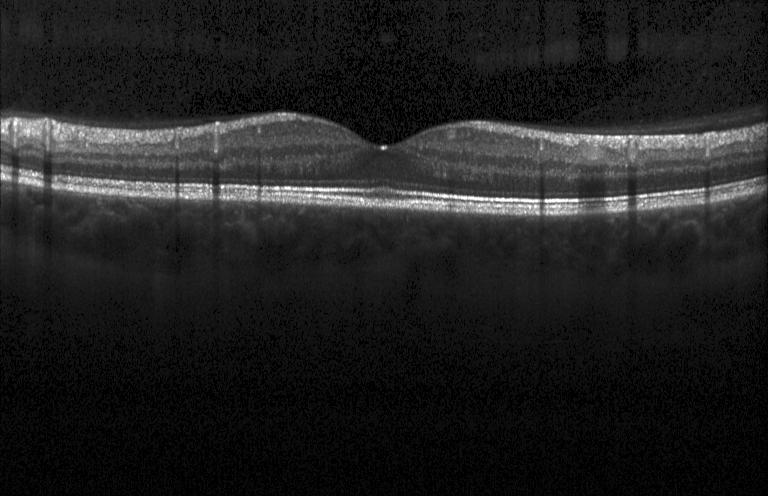

OCT line scan.
Macular OCT: no CNV, DME, or drusen.